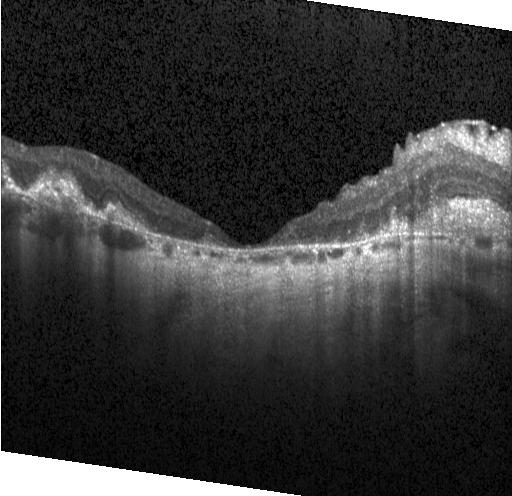
Optical coherence tomography B-scan. Impression: CNV.